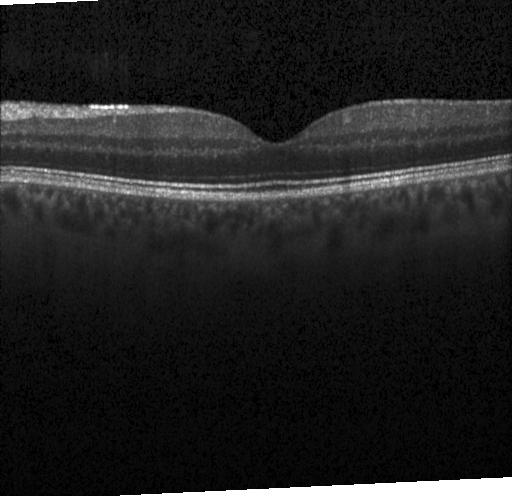

Centered on the fovea · SD-OCT · OCT line scan. No choroidal neovascularization, diabetic macular edema, or drusen.